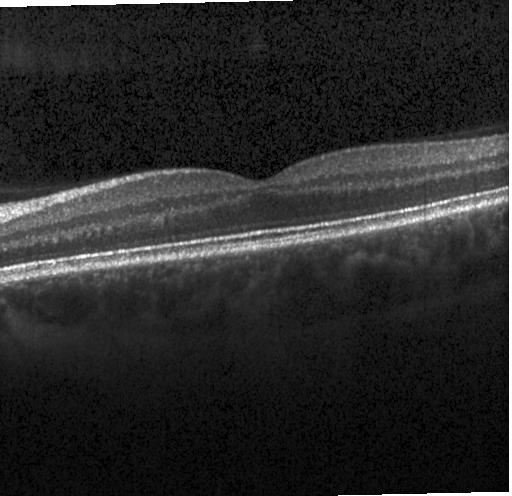

Optical coherence tomography scan
OCT finding: neither choroidal neovascularization, diabetic macular edema, nor drusen.